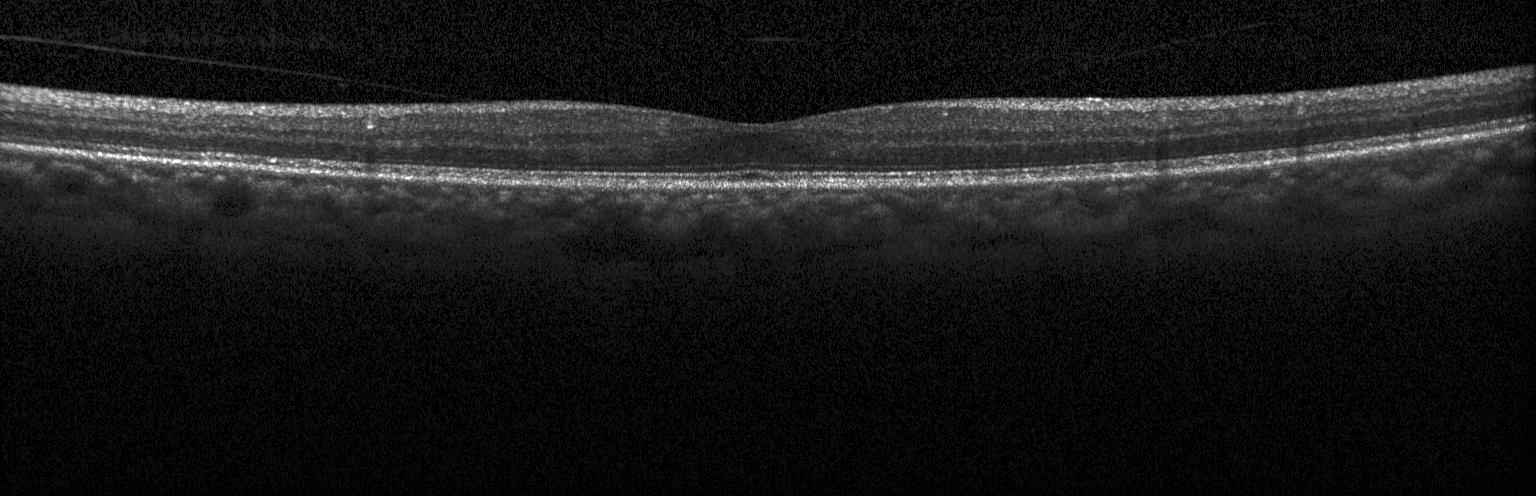 Diagnosis: no choroidal neovascularization, diabetic macular edema, or drusen.